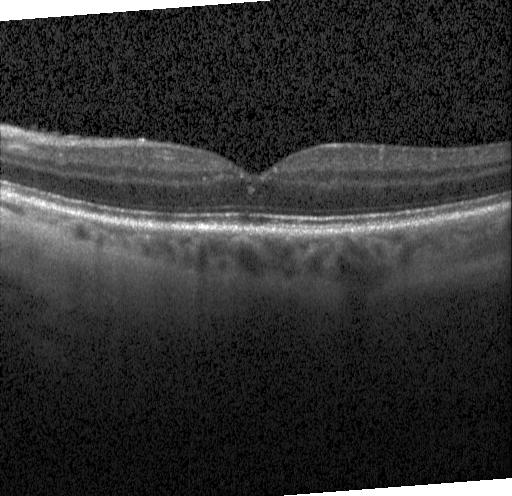

Retinal OCT cross-section. Acquired on a Heidelberg Spectralis — Macular OCT: no CNV, DME, or drusen.